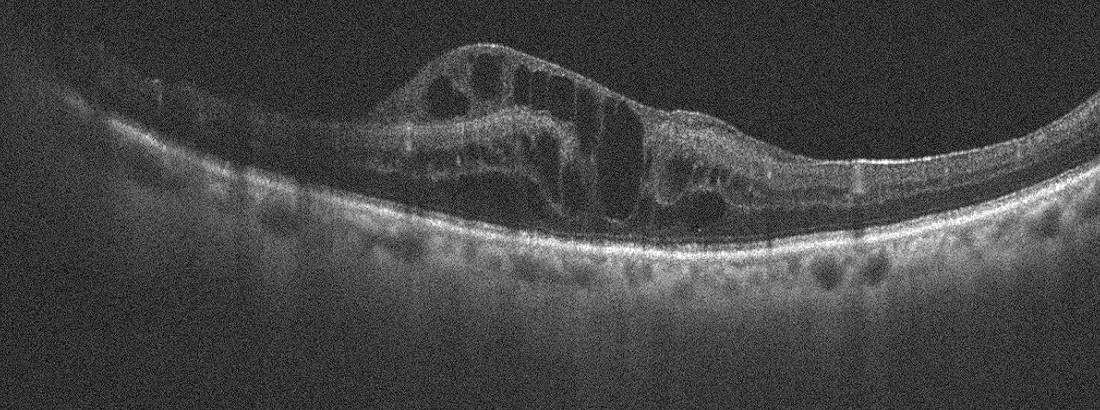
OCT B-scan. Optovue Avanti RTVue XR — Impression: retinal vein occlusion.